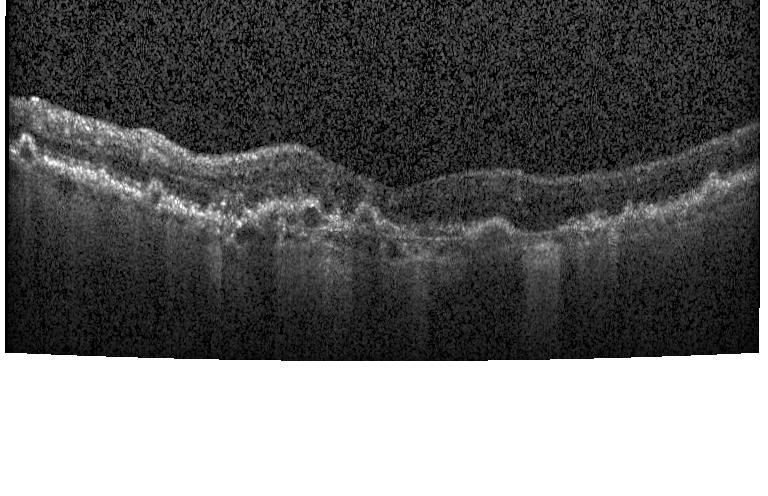 OCT B-scan; fovea-centered
Finding: choroidal neovascularization.